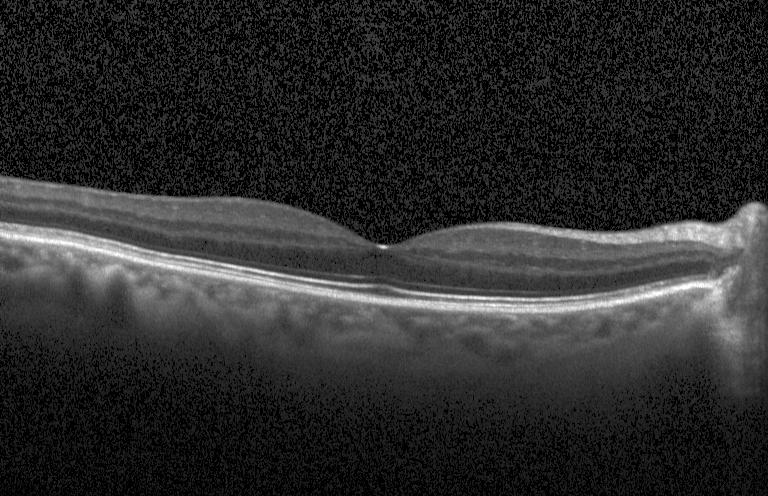

Macular OCT demonstrating no choroidal neovascularization, diabetic macular edema, or drusen.